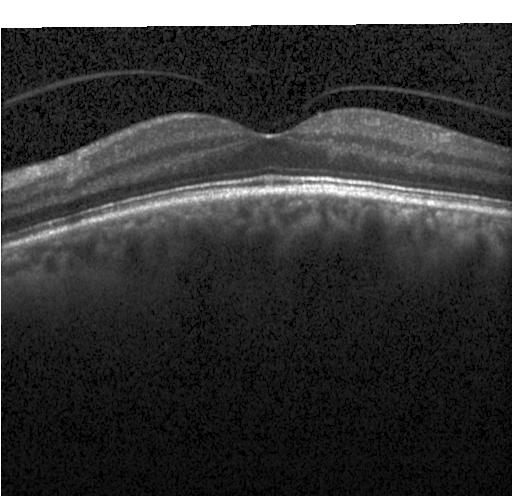

Retinal OCT cross-section showing neither choroidal neovascularization, diabetic macular edema, nor drusen.